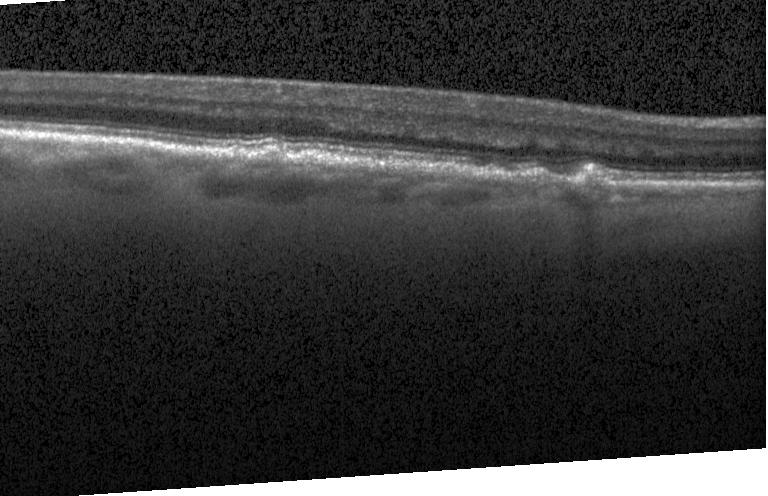
Impression: drusen.